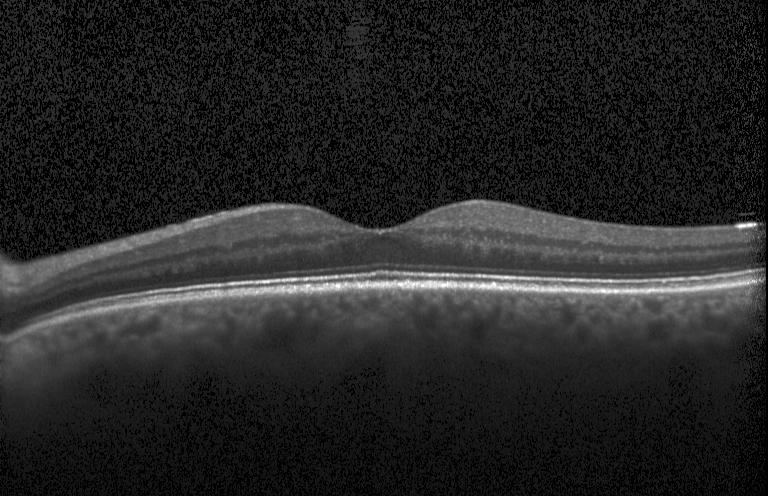 Impression: no evidence of choroidal neovascularization, diabetic macular edema, or drusen.